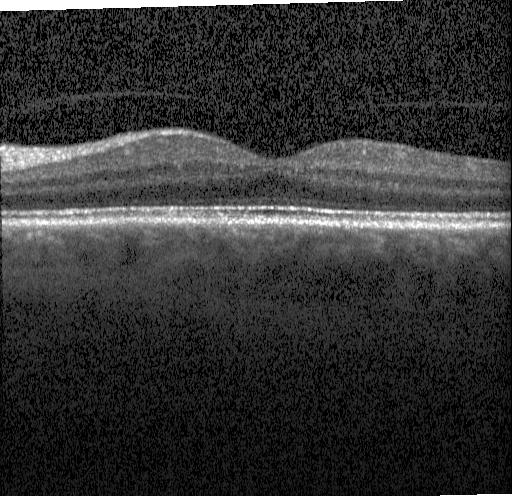
Macular OCT demonstrating no choroidal neovascularization, no diabetic macular edema, and no drusen.